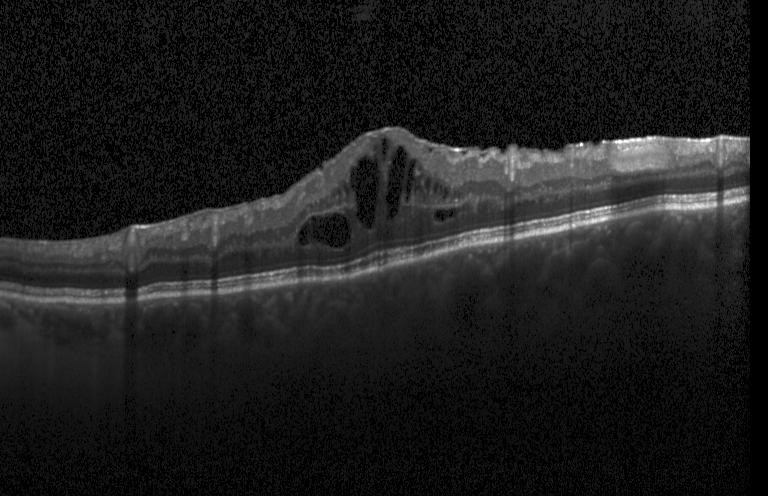

Optical coherence tomography B-scan · fovea-centered · instrument: Heidelberg Spectralis — The scan shows diabetic macular edema.